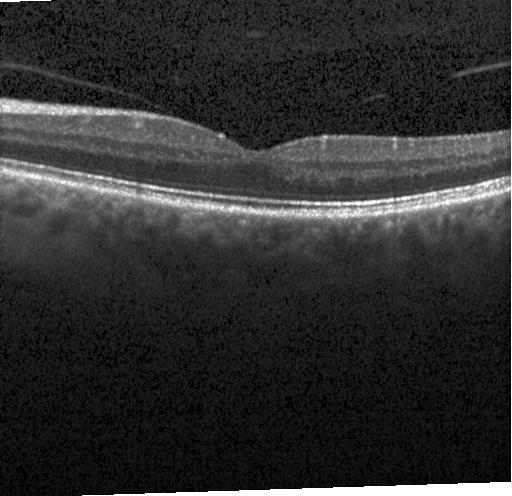

Finding: no evidence of choroidal neovascularization, diabetic macular edema, or drusen.